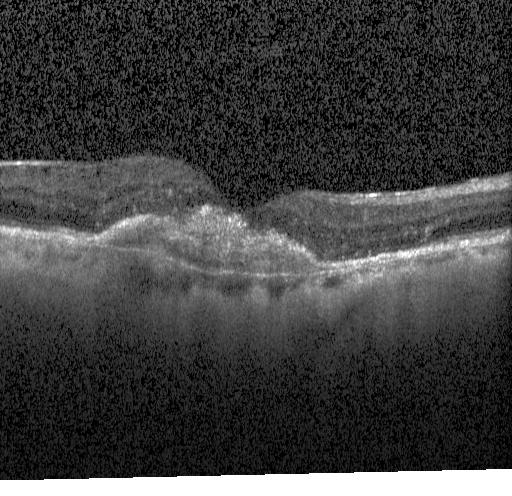 Impression: choroidal neovascularization (CNV).